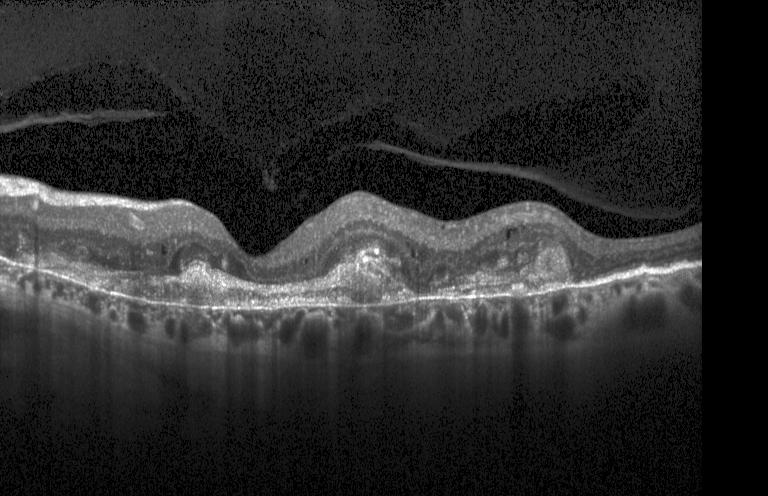 Through the macula, spectral-domain OCT, Heidelberg Spectralis, retinal OCT cross-section
Macular OCT: a choroidal neovascular membrane.